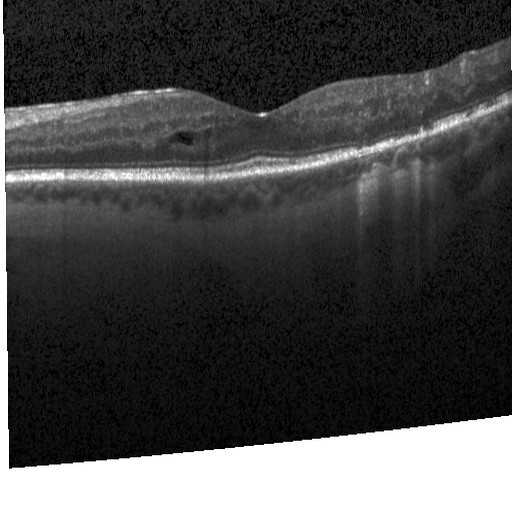
Assessment: diabetic macular edema (DME).